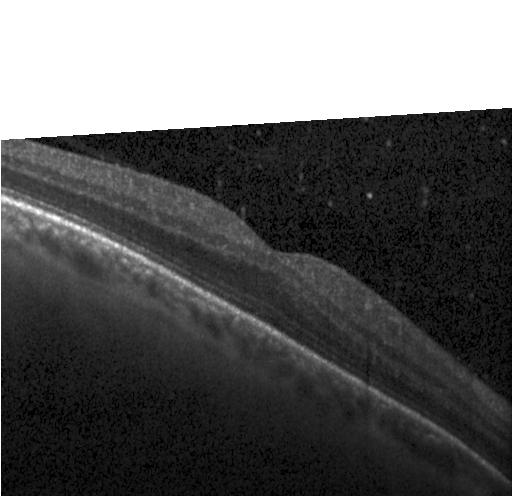 Retinal OCT B-scan. Spectral-domain optical coherence tomography. Heidelberg Spectralis OCT system. Centered on the fovea. Diagnosis: no CNV, DME, or drusen.